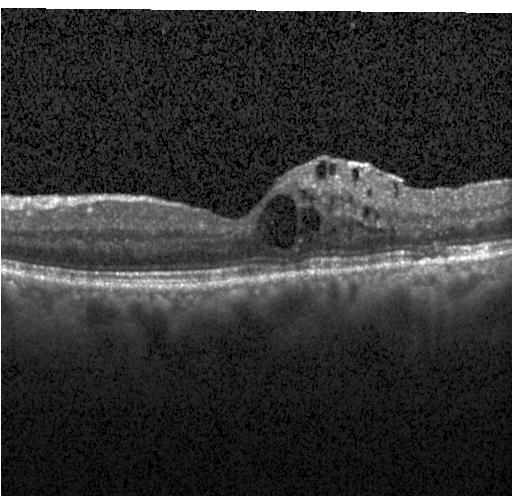 OCT line scan
Impression: diabetic macular edema.